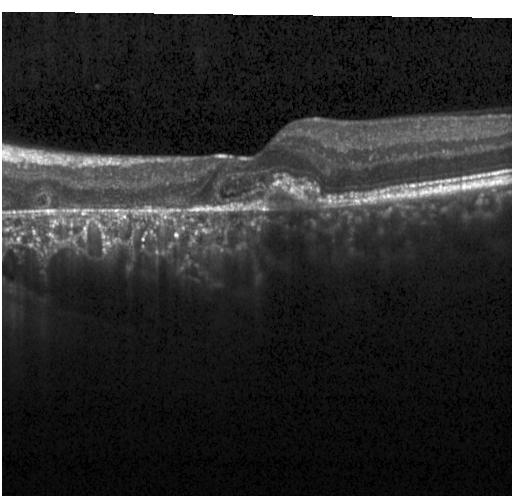
The scan shows CNV.